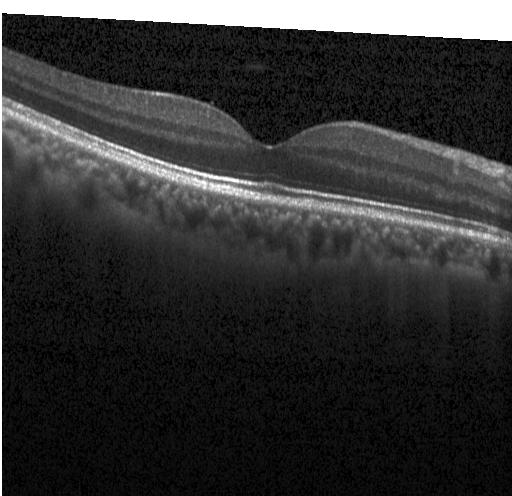

Dx: no choroidal neovascularization, no diabetic macular edema, and no drusen.